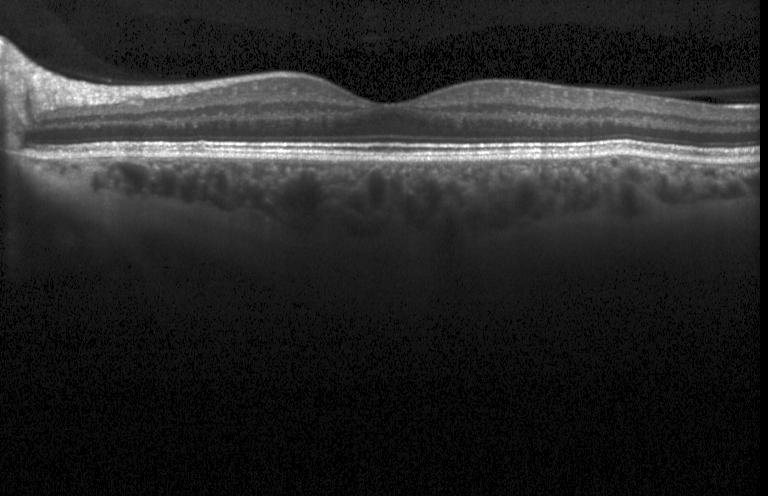 OCT line scan. Diagnosis: neither choroidal neovascularization, diabetic macular edema, nor drusen.